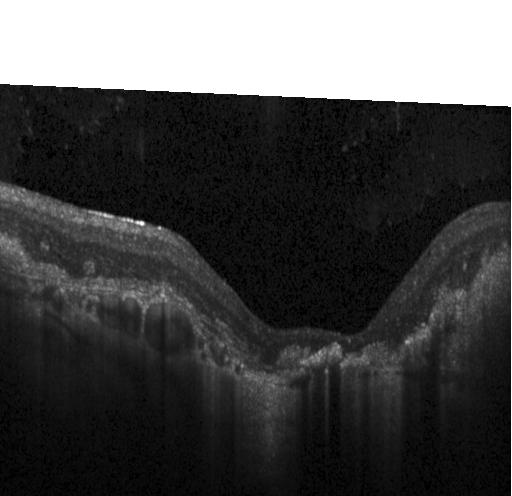

The scan shows a choroidal neovascular membrane.